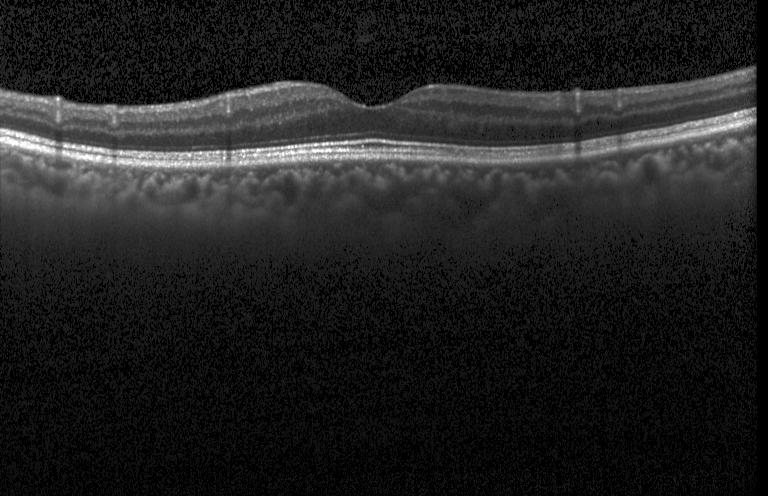

Through the macula. OCT line scan. Heidelberg Spectralis
Finding: no evidence of choroidal neovascularization, diabetic macular edema, or drusen.